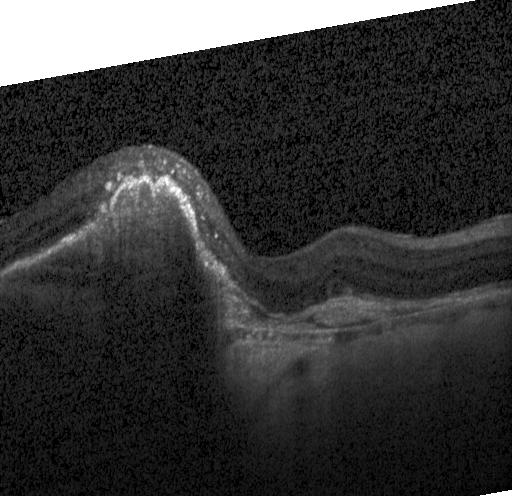
The scan shows CNV.